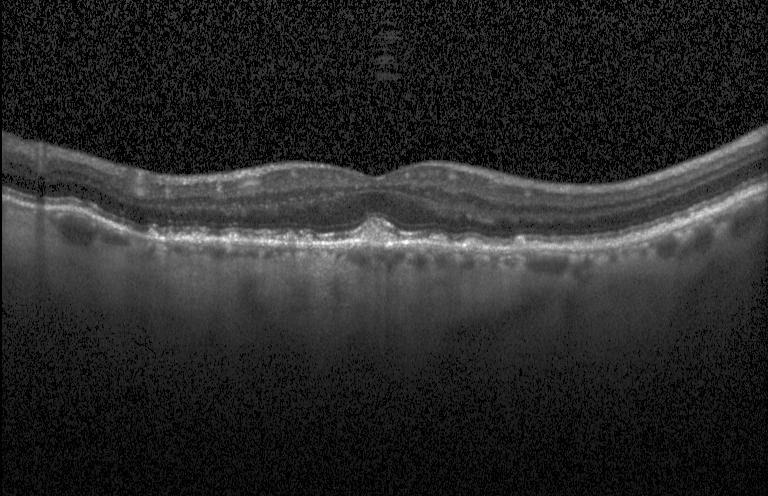

Macular scan; OCT B-scan; spectral-domain OCT — Dx: drusen.